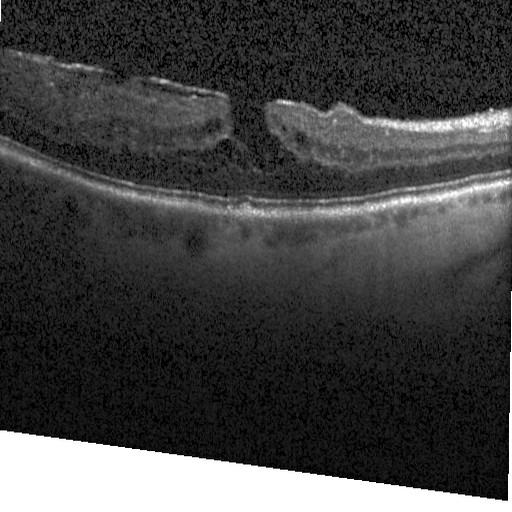 Through the macula, OCT line scan
Finding: DME.